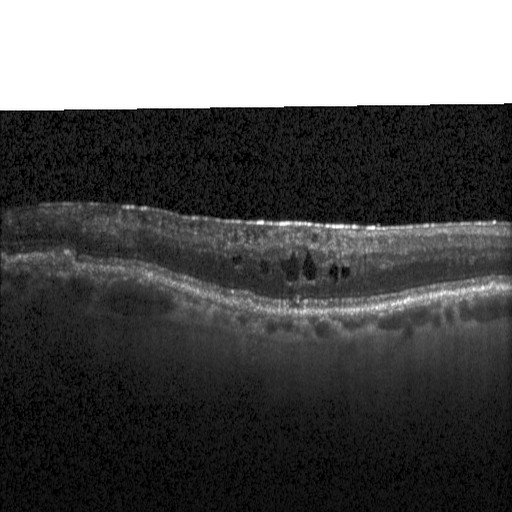
Diagnosis: DME.